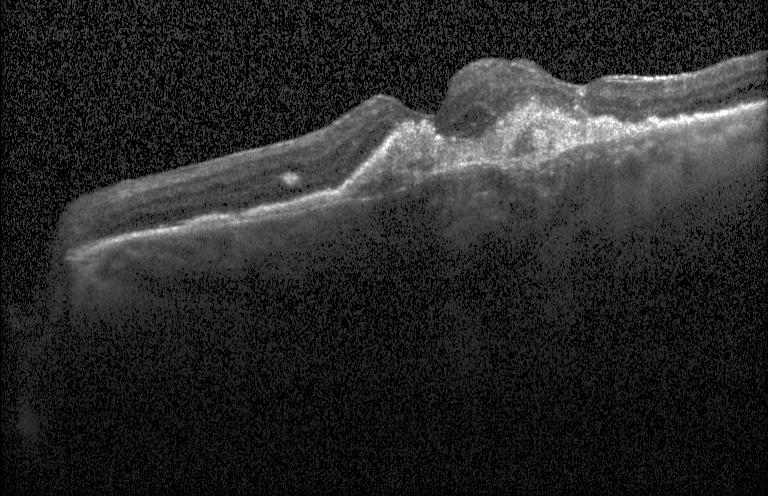
Macular scan · retinal OCT cross-section
Dx: a choroidal neovascular membrane.